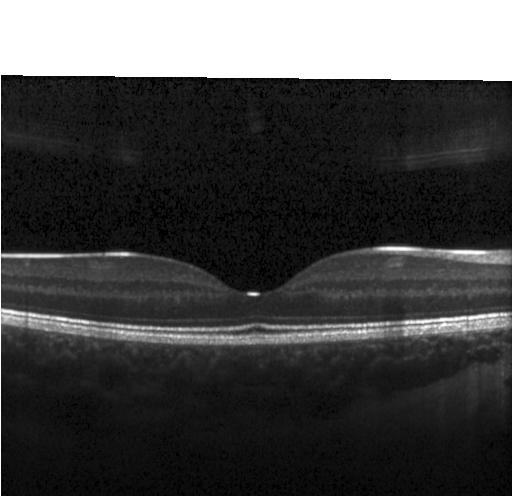 Macular OCT: no choroidal neovascularization, diabetic macular edema, or drusen.